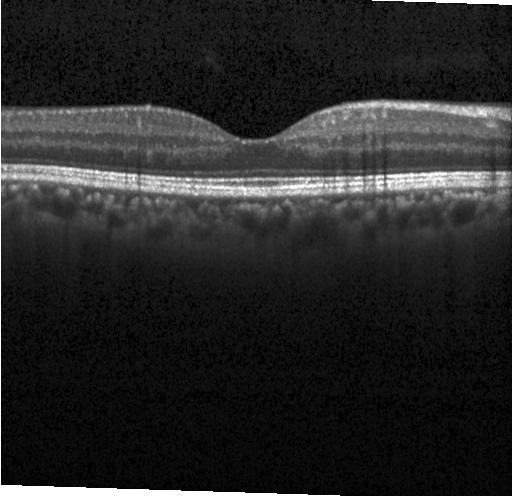 Spectral-domain OCT. Optical coherence tomography B-scan
OCT finding: no choroidal neovascularization, no diabetic macular edema, and no drusen.